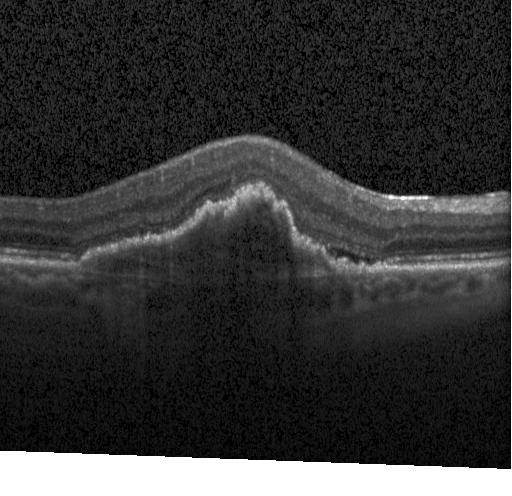
Optical coherence tomography scan; Heidelberg Spectralis OCT system — A choroidal neovascular membrane.